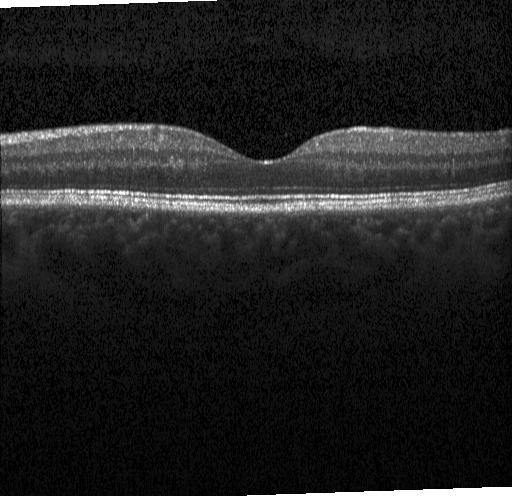

Retinal OCT cross-section, instrument: Heidelberg Spectralis, macular scan
Impression: no choroidal neovascularization, diabetic macular edema, or drusen.